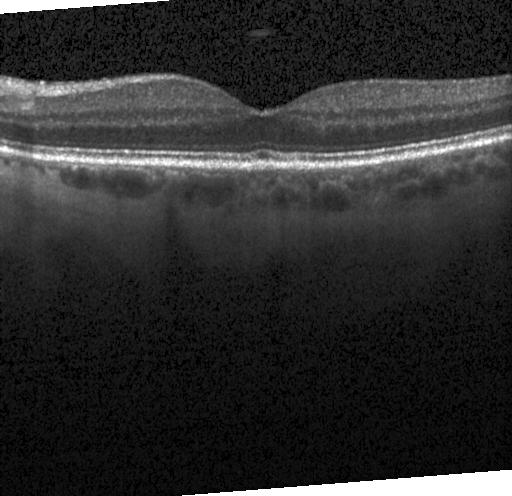 SD-OCT; optical coherence tomography B-scan; fovea-centered; instrument: Heidelberg Spectralis. No evidence of choroidal neovascularization, diabetic macular edema, or drusen.